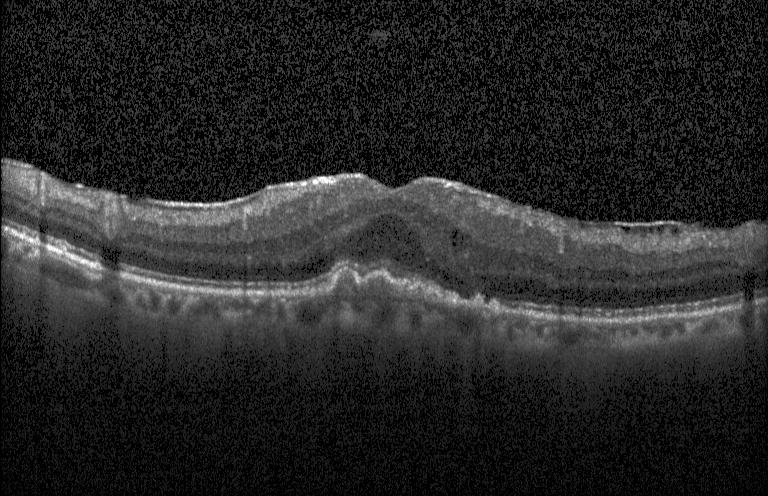
Retinal OCT cross-section showing a choroidal neovascular membrane.